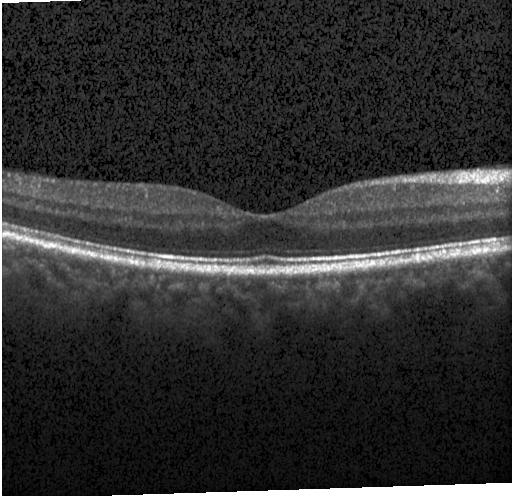
OCT line scan. OCT finding: no CNV, DME, or drusen.